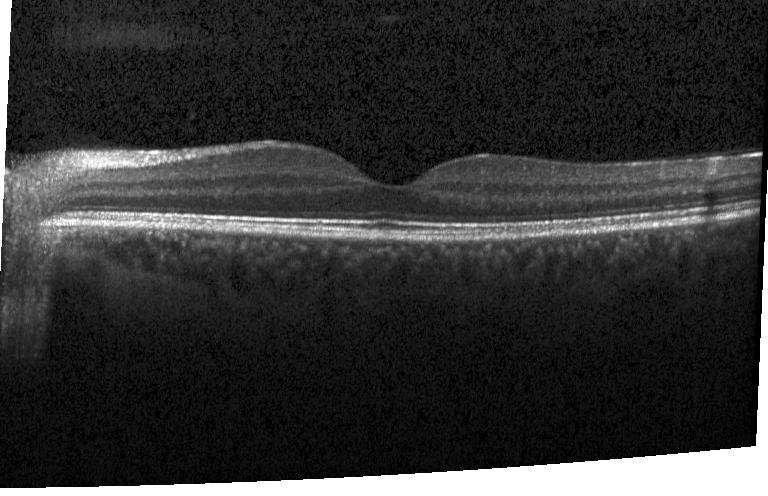

OCT scan showing no CNV, DME, or drusen.